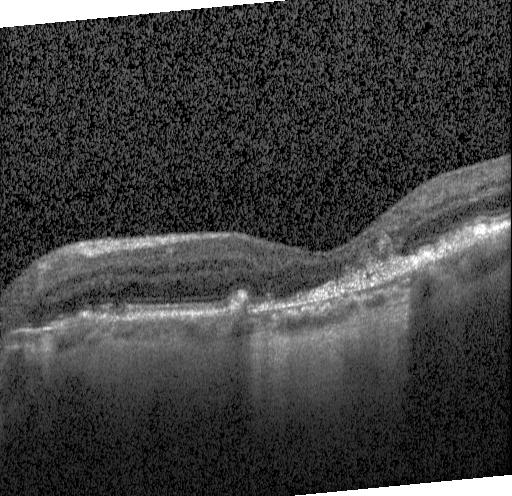 SD-OCT, OCT line scan
Assessment: a choroidal neovascular membrane.